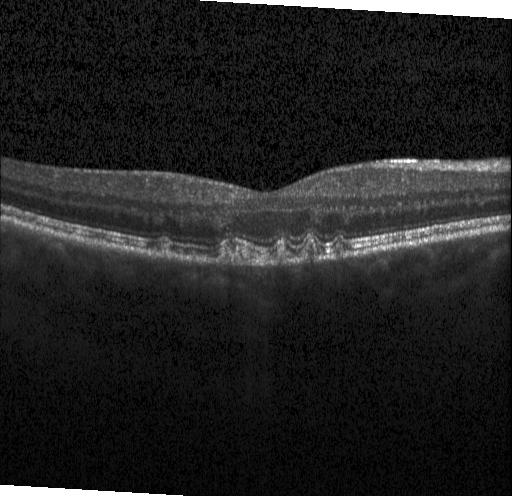
OCT B-scan; Heidelberg Spectralis; SD-OCT; centered on the fovea.
Assessment: multiple drusen.